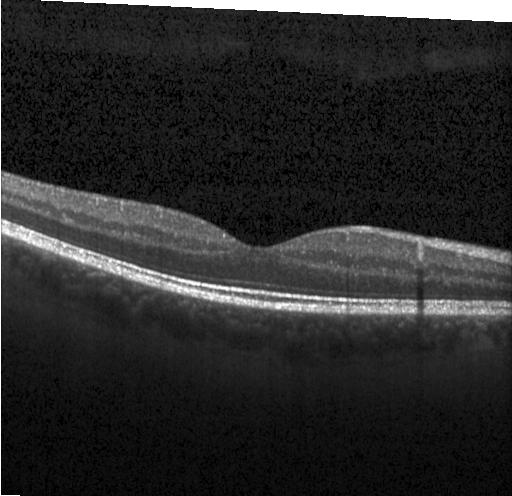
Macular OCT demonstrating no CNV, DME, or drusen.